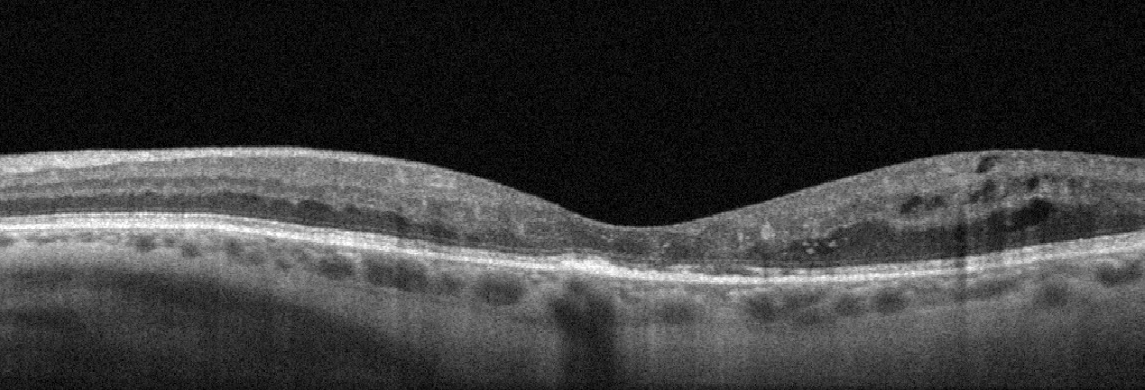 Retinal OCT B-scan
Diagnosis: DME.